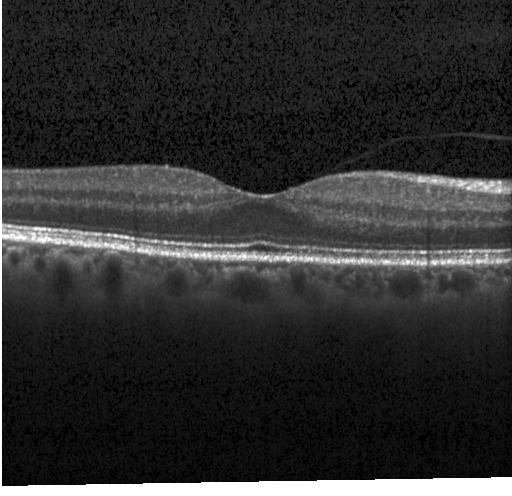

This B-scan demonstrates no evidence of choroidal neovascularization, diabetic macular edema, or drusen.